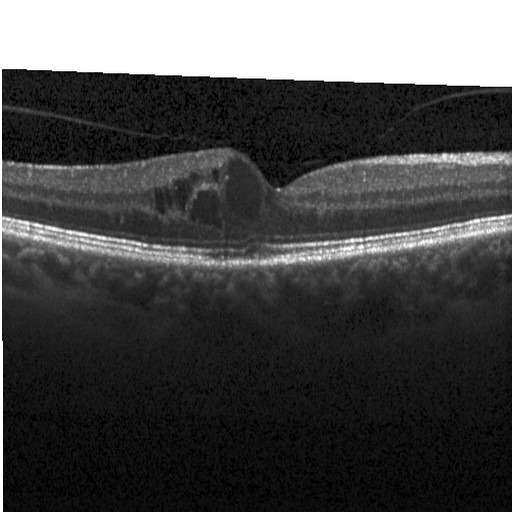 Impression: DME.